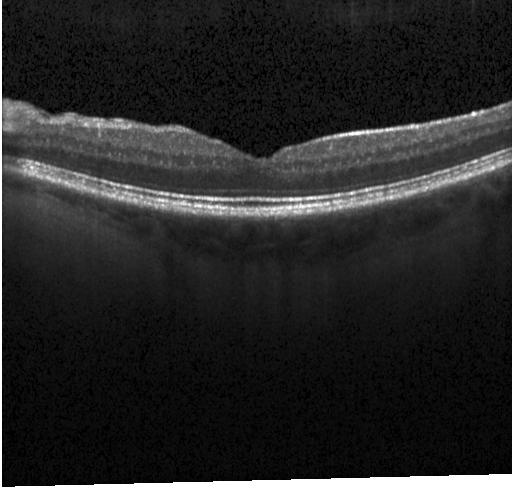 Diagnosis: no evidence of choroidal neovascularization, diabetic macular edema, or drusen.